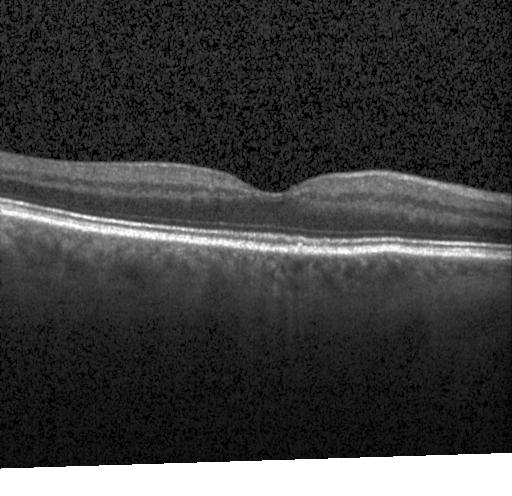
OCT B-scan. Heidelberg Spectralis. Impression: no evidence of choroidal neovascularization, diabetic macular edema, or drusen.